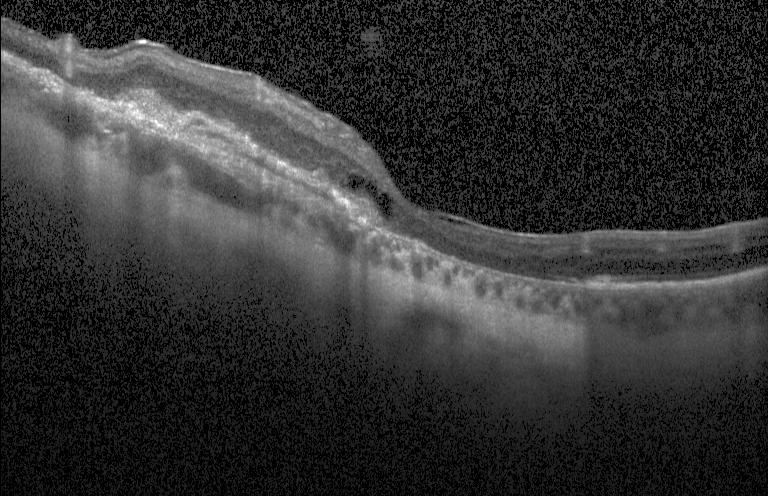

Impression: a choroidal neovascular membrane.